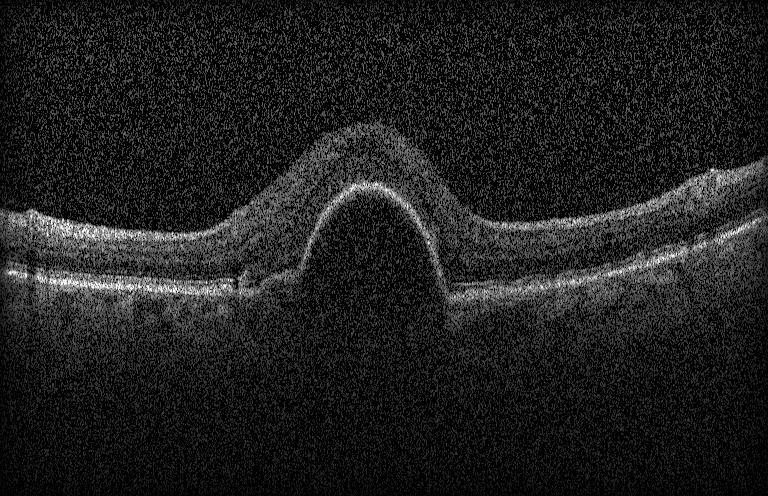
Retinal OCT B-scan; horizontal scan through the fovea; acquired on a Heidelberg Spectralis.
The scan shows a choroidal neovascular membrane.